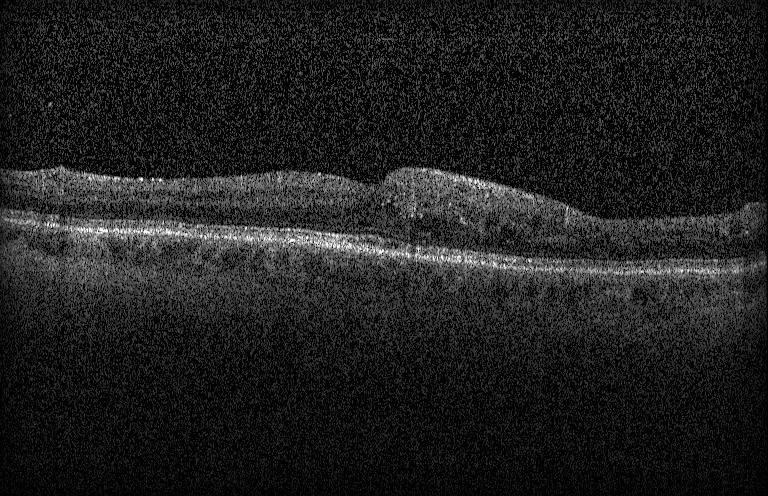 The scan shows diabetic macular edema (DME).